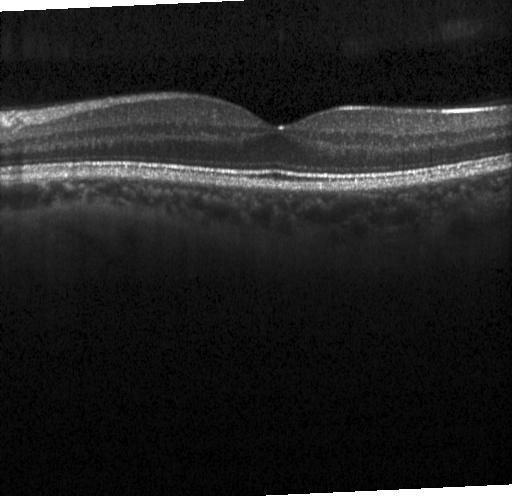
OCT scan showing no evidence of CNV, DME, or drusen.